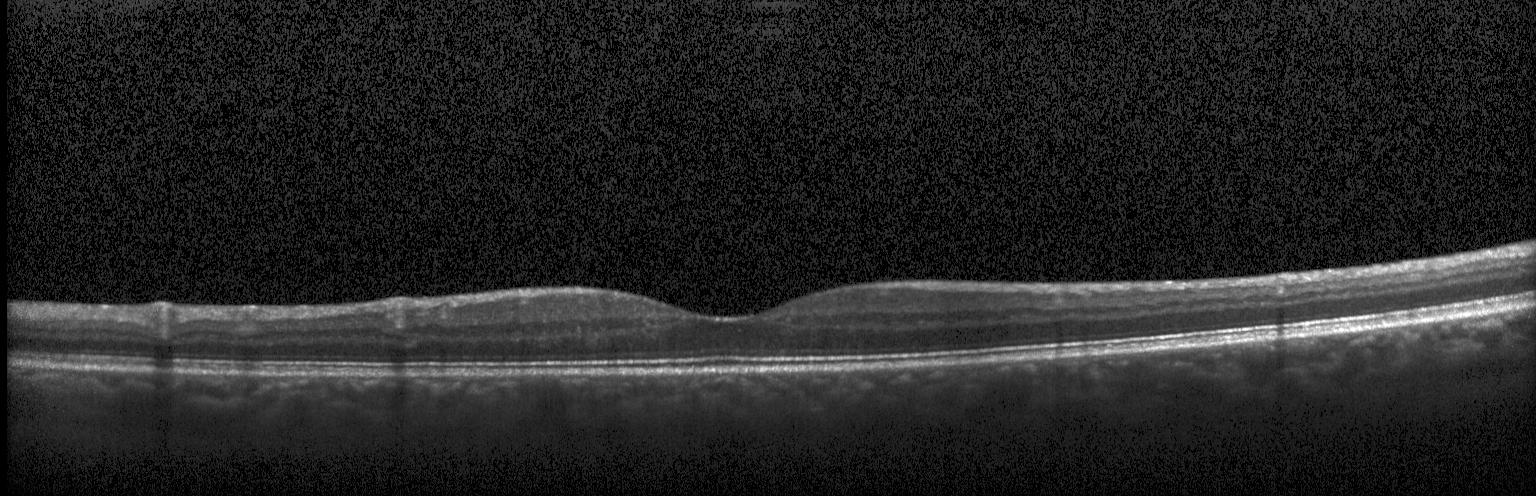
Spectral-domain OCT, acquired on a Heidelberg Spectralis, optical coherence tomography scan, macular scan — Finding: no choroidal neovascularization, no diabetic macular edema, and no drusen.